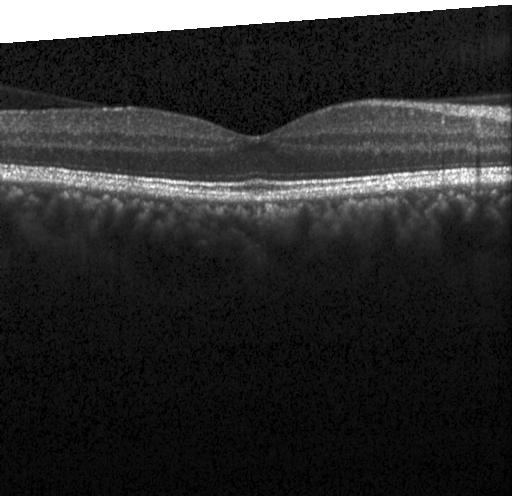
Impression: no choroidal neovascularization, diabetic macular edema, or drusen.